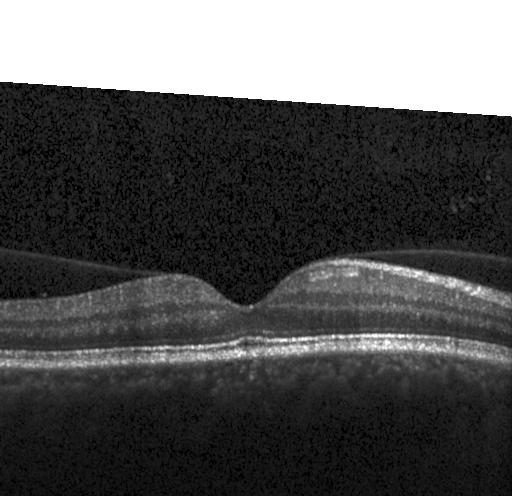 Finding: no CNV, no DME, and no drusen.